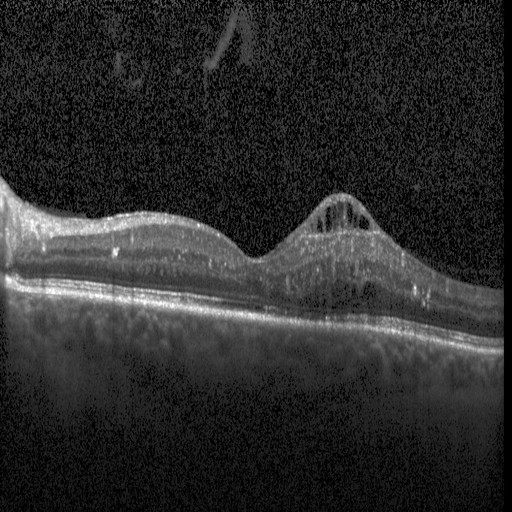 Centered on the fovea. OCT line scan. SD-OCT.
This B-scan demonstrates diabetic macular edema (DME).